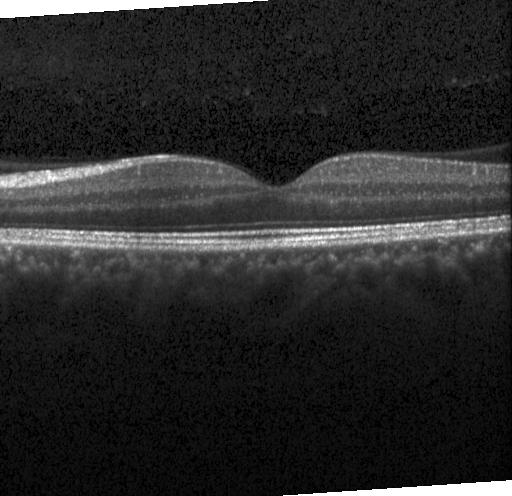

SD-OCT. Retinal OCT B-scan. Centered on the fovea. This B-scan demonstrates no evidence of CNV, DME, or drusen.